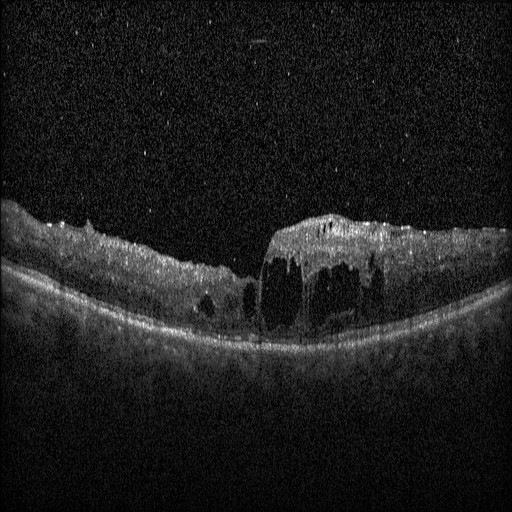 OCT finding: diabetic macular edema.